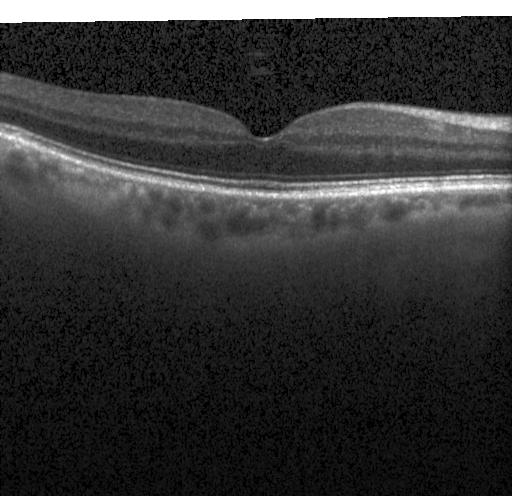

SD-OCT · optical coherence tomography scan — Finding: no choroidal neovascularization, no diabetic macular edema, and no drusen.